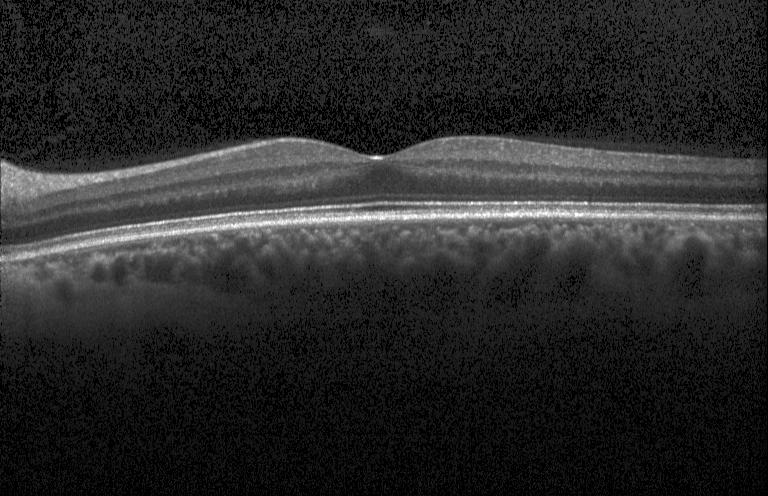 Optical coherence tomography scan · spectral-domain OCT · Heidelberg Spectralis OCT system
Impression: no choroidal neovascularization, diabetic macular edema, or drusen.